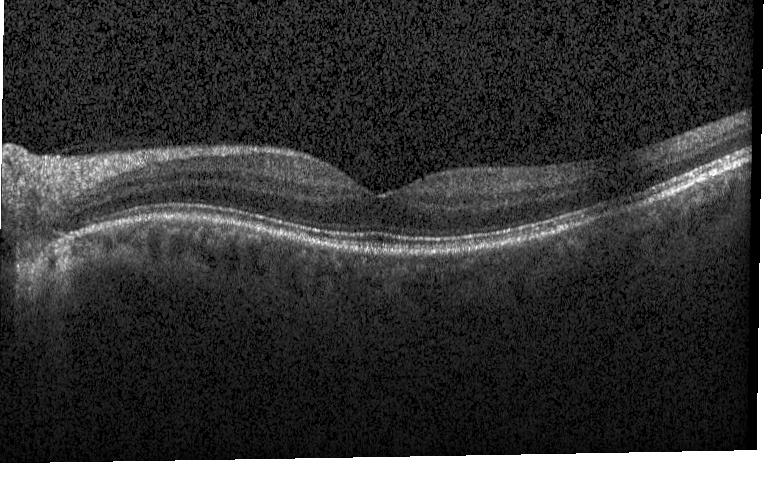 Optical coherence tomography B-scan · SD-OCT · through the macula. No evidence of choroidal neovascularization, diabetic macular edema, or drusen.